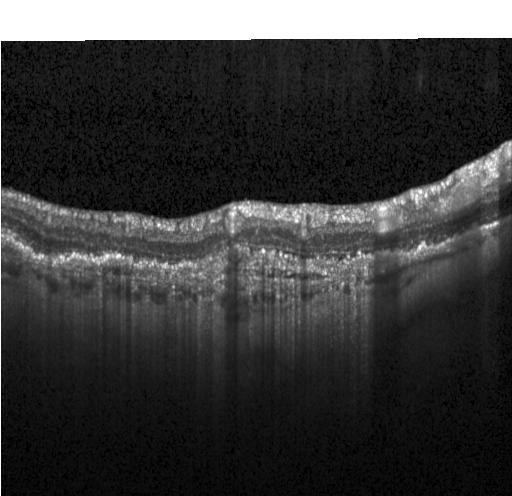

Spectral-domain OCT · OCT B-scan · horizontal scan through the fovea · Heidelberg Spectralis.
The scan shows a choroidal neovascular membrane.